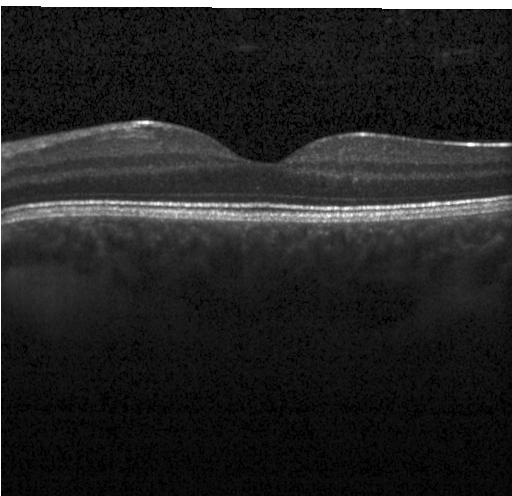 Optical coherence tomography B-scan. Heidelberg Spectralis. Macular scan. SD-OCT
Finding: neither choroidal neovascularization, diabetic macular edema, nor drusen.